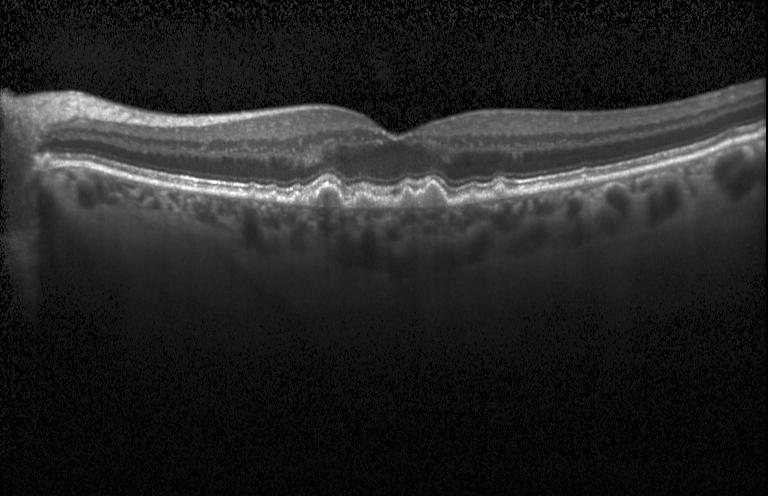

Horizontal scan through the fovea; retinal OCT cross-section.
OCT finding: drusen.